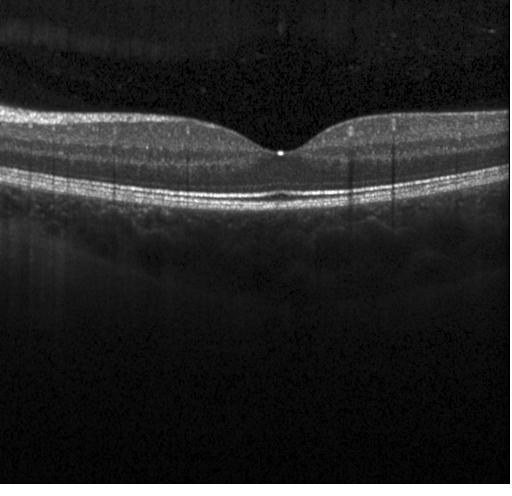

SD-OCT, Heidelberg Spectralis, fovea-centered, optical coherence tomography B-scan.
Macular OCT: no choroidal neovascularization, diabetic macular edema, or drusen.